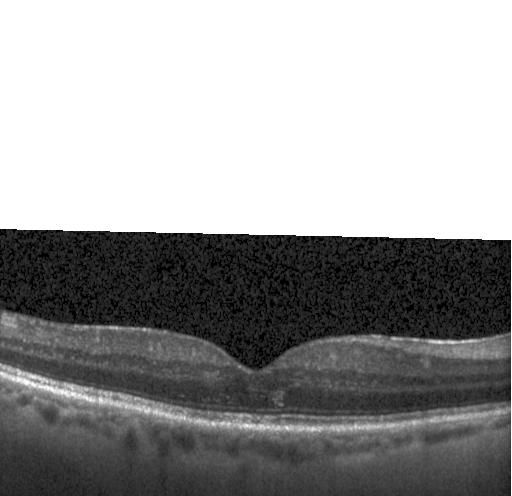 Retinal OCT B-scan. Macular OCT: no evidence of CNV, DME, or drusen.